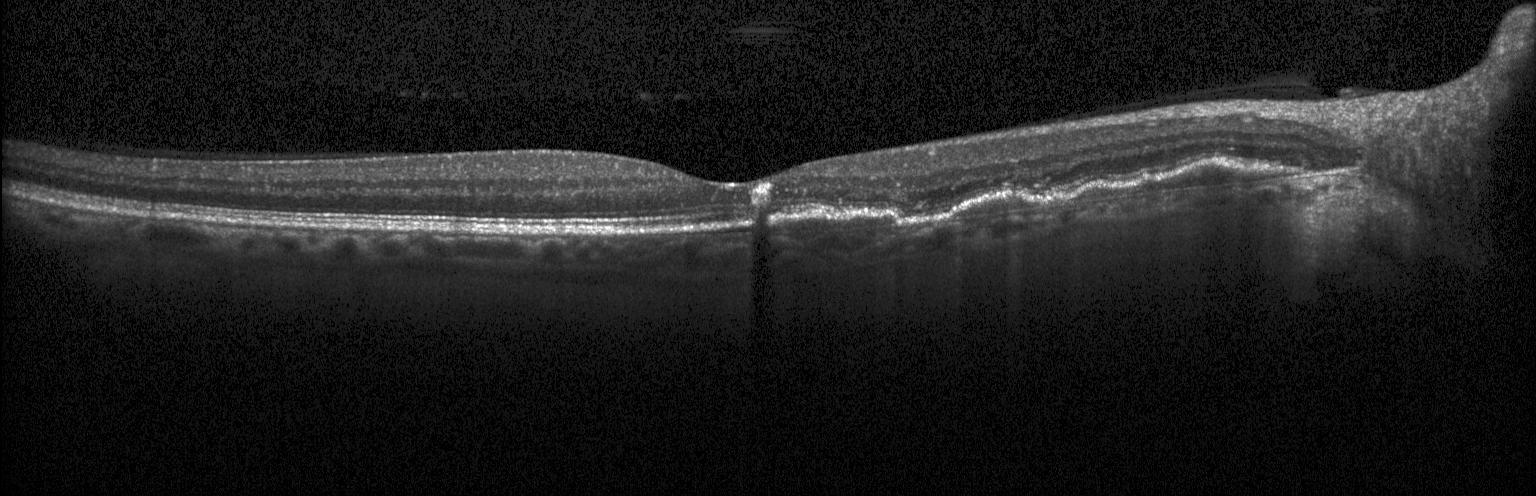

Finding: a choroidal neovascular membrane.